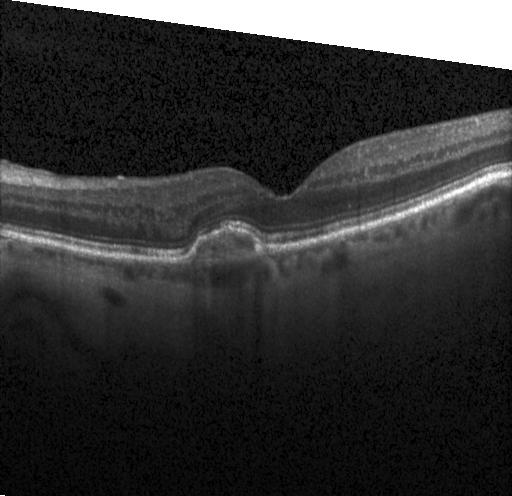 Spectral-domain OCT · Heidelberg Spectralis OCT system · optical coherence tomography scan — Finding: choroidal neovascularization (CNV).